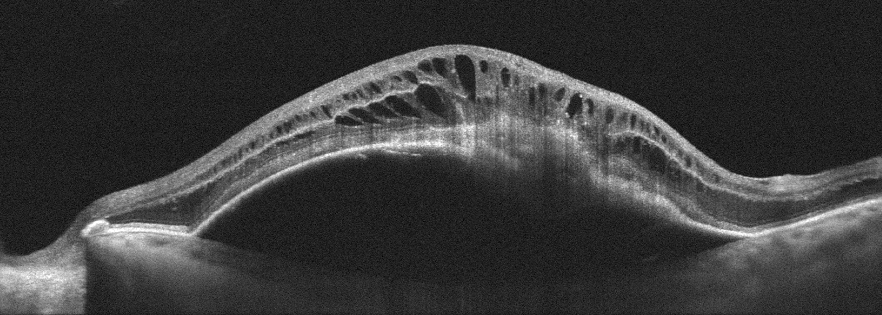
OCT B-scan, instrument: Optovue Avanti RTVue XR.
Impression: age-related macular degeneration (AMD).